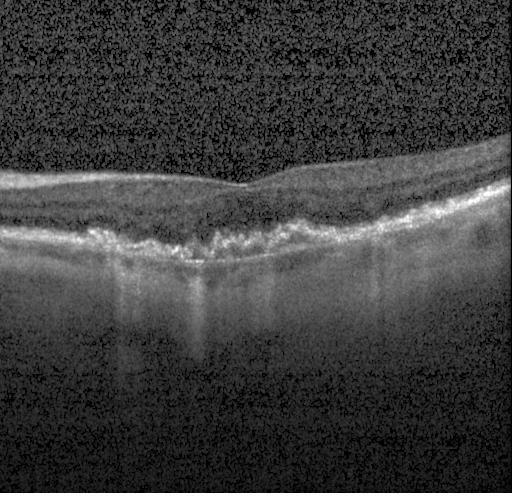 Retinal OCT B-scan
This B-scan demonstrates CNV.